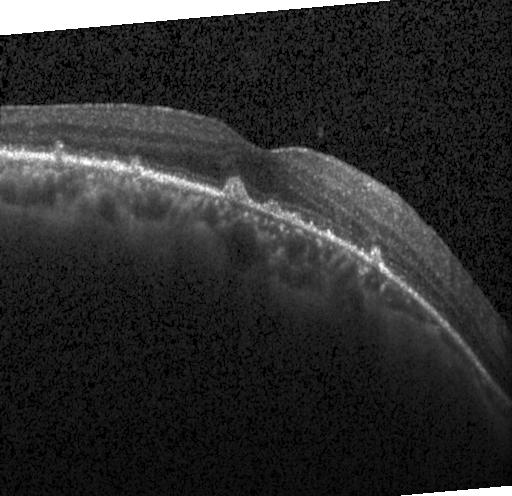
Retinal OCT B-scan.
Diagnosis: drusen.